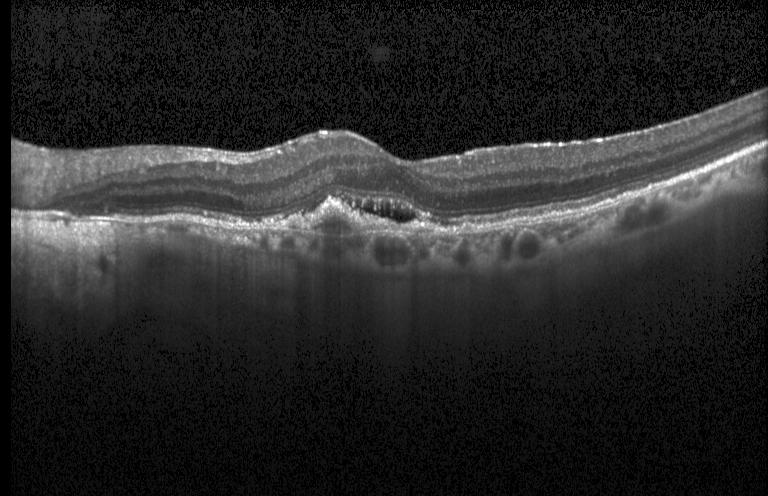

Centered on the fovea · optical coherence tomography scan · instrument: Heidelberg Spectralis
The scan shows a choroidal neovascular membrane.